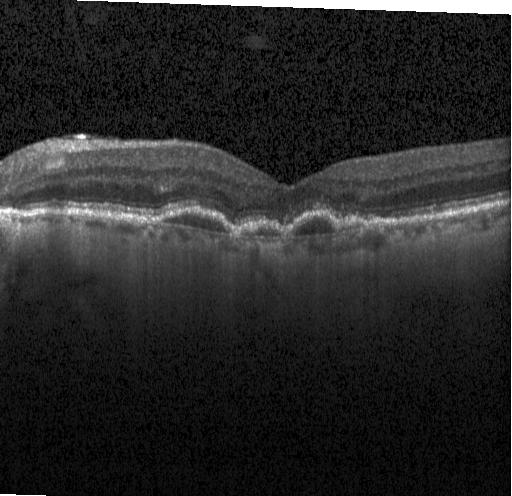

Spectral-domain optical coherence tomography, macular scan, retinal OCT B-scan — OCT finding: a choroidal neovascular membrane.